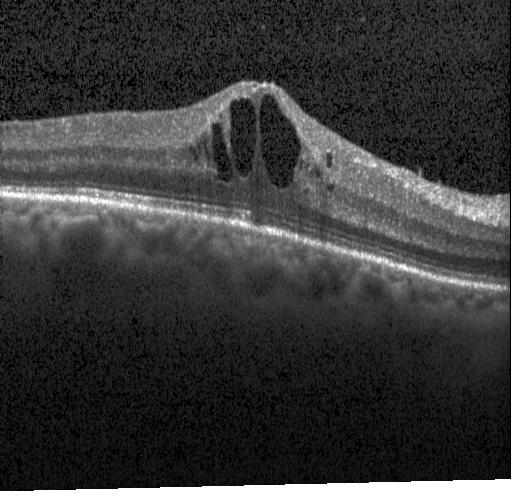
Optical coherence tomography B-scan. Impression: diabetic macular edema.